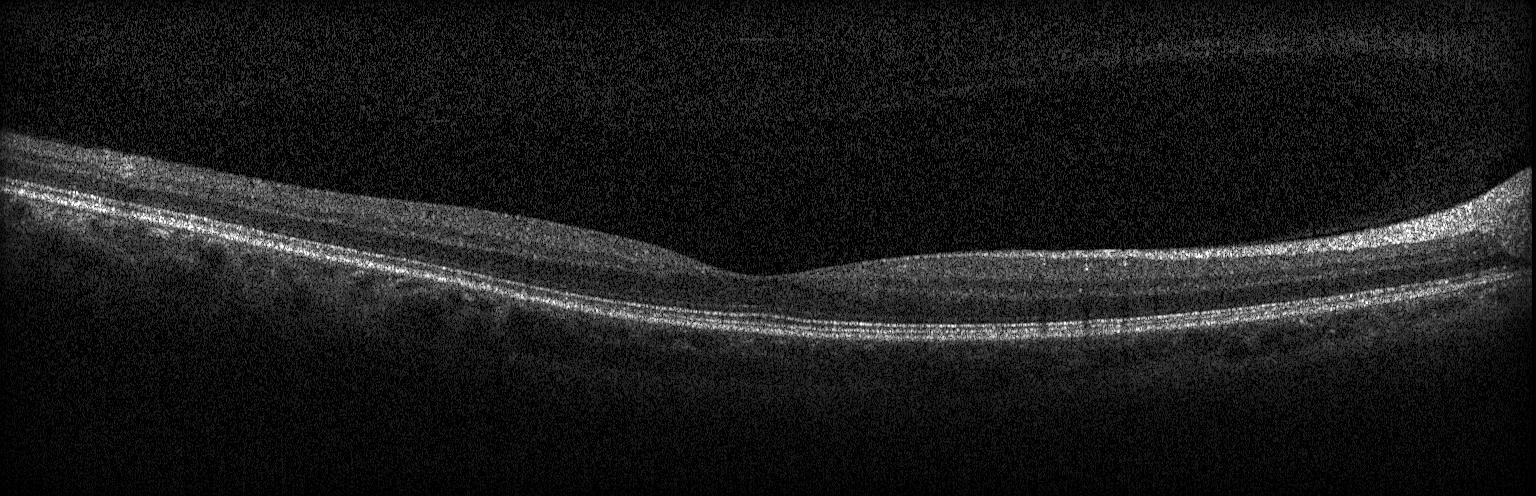 Optical coherence tomography scan · spectral-domain OCT · fovea-centered. Diagnosis: no choroidal neovascularization, diabetic macular edema, or drusen.